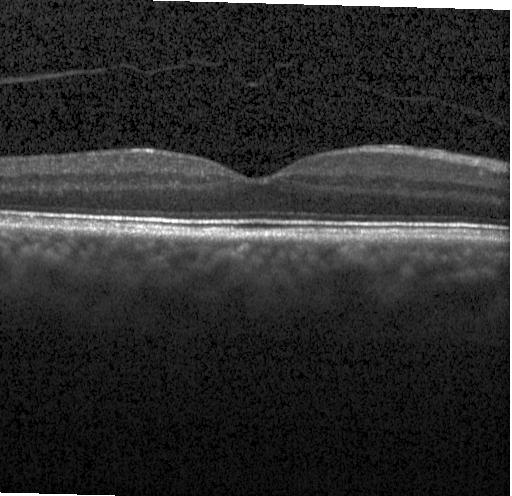
Optical coherence tomography scan, fovea-centered
OCT finding: no choroidal neovascularization, diabetic macular edema, or drusen.